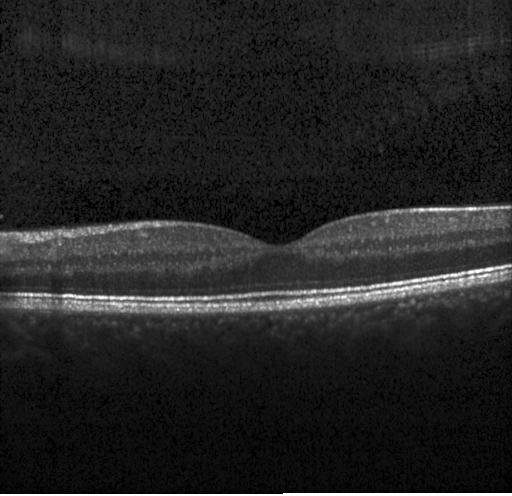

OCT line scan · instrument: Heidelberg Spectralis
Impression: no choroidal neovascularization, diabetic macular edema, or drusen.